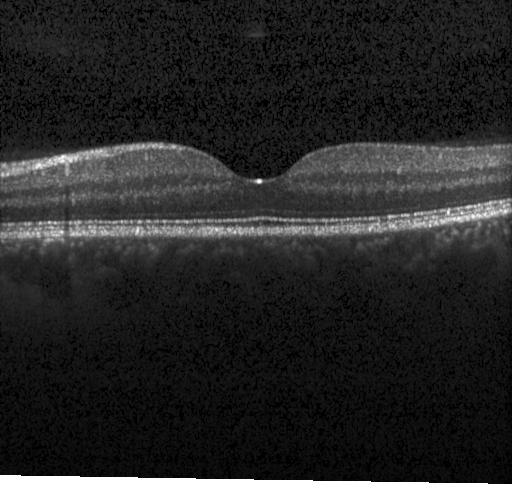

Dx: neither CNV, DME, nor drusen.